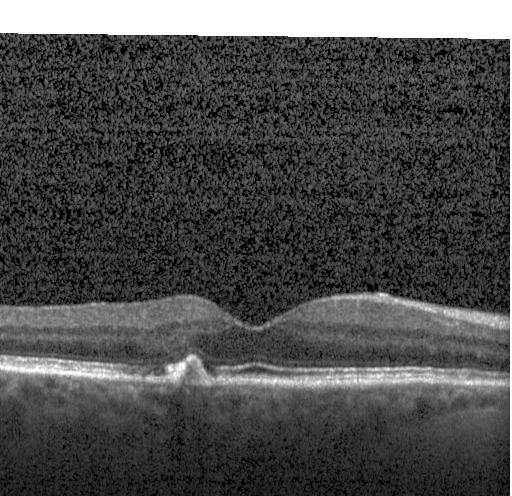
Macular OCT demonstrating multiple drusen.